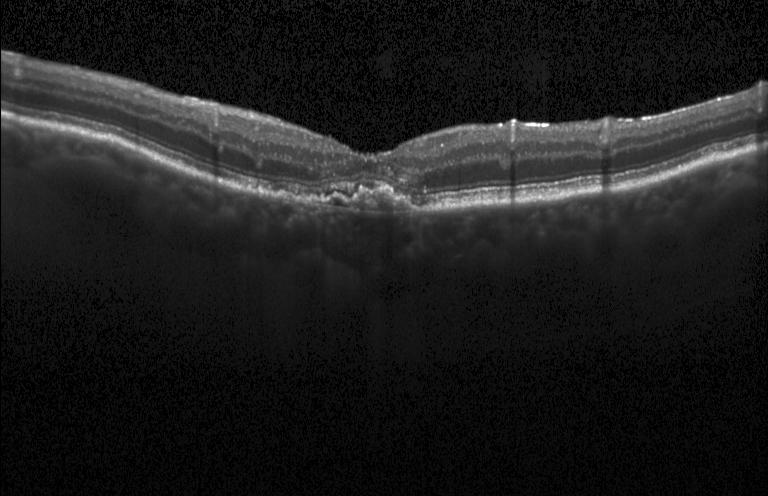

Centered on the fovea. Retinal OCT cross-section. SD-OCT
This B-scan demonstrates a choroidal neovascular membrane.